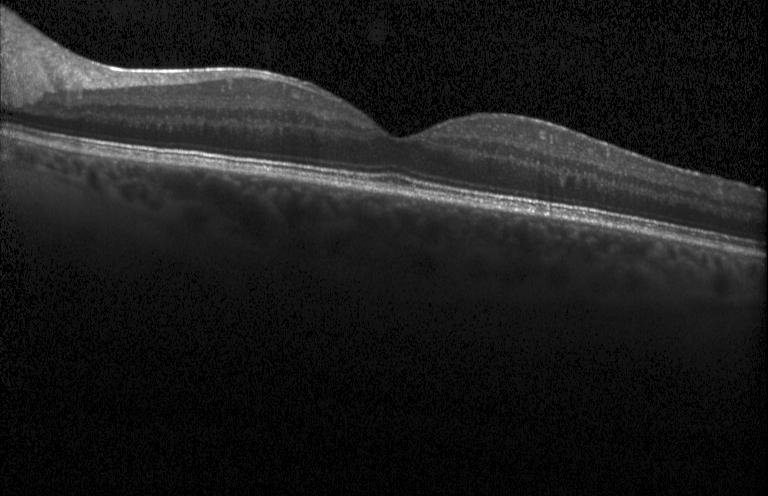 Macular OCT: no choroidal neovascularization, no diabetic macular edema, and no drusen.